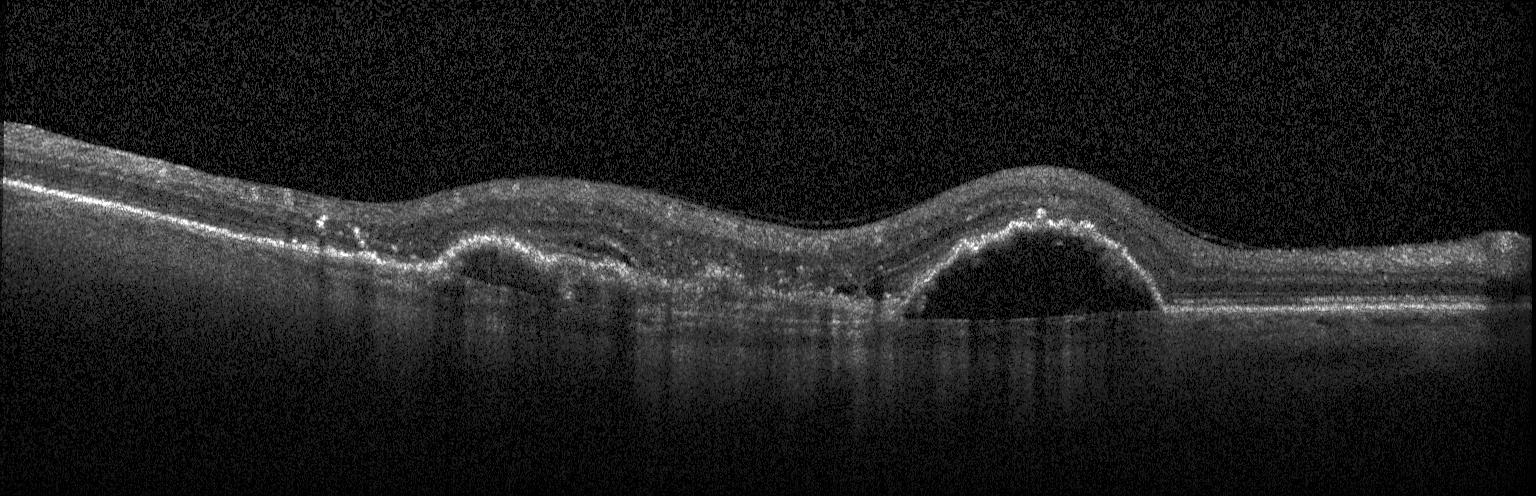

Centered on the fovea, Heidelberg Spectralis, OCT line scan, SD-OCT
Impression: choroidal neovascularization (CNV).